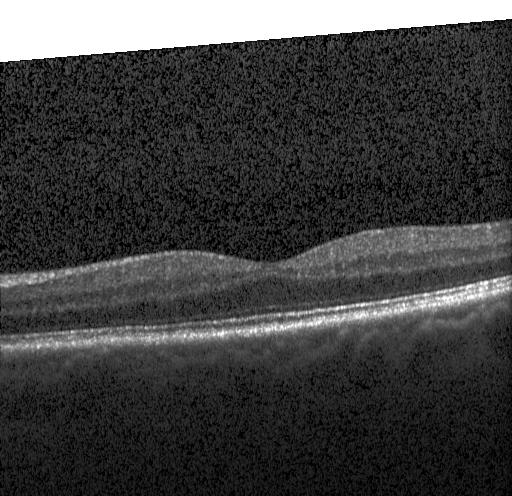
Retinal OCT cross-section; spectral-domain optical coherence tomography; Heidelberg Spectralis OCT system — Finding: neither choroidal neovascularization, diabetic macular edema, nor drusen.